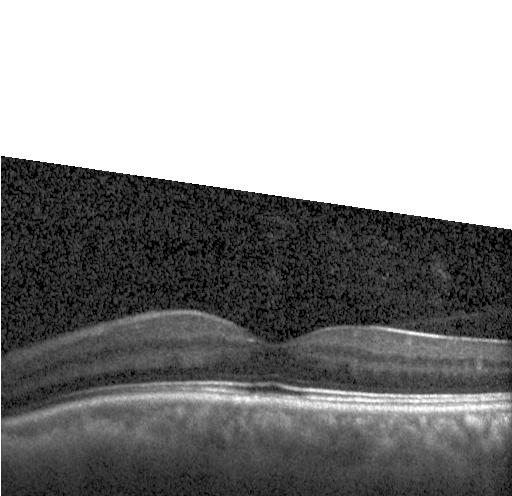 Diagnosis: neither CNV, DME, nor drusen.